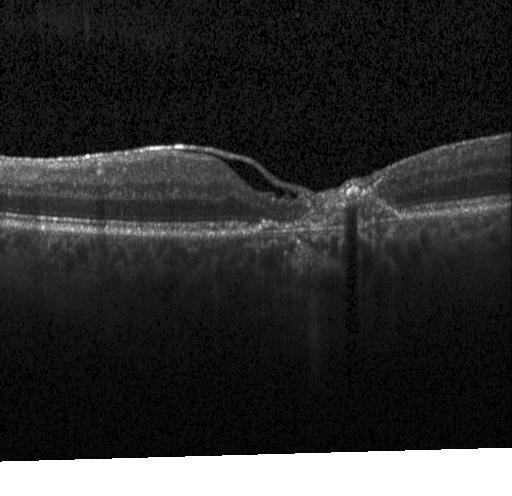 Choroidal neovascularization (CNV).